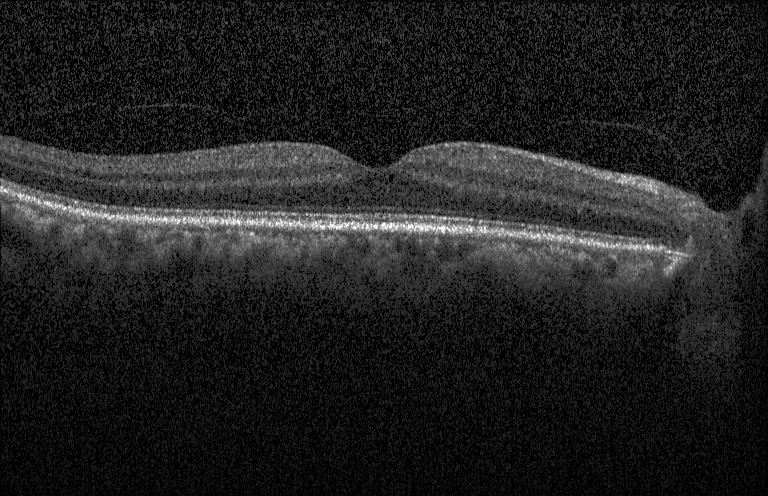

No choroidal neovascularization, diabetic macular edema, or drusen.